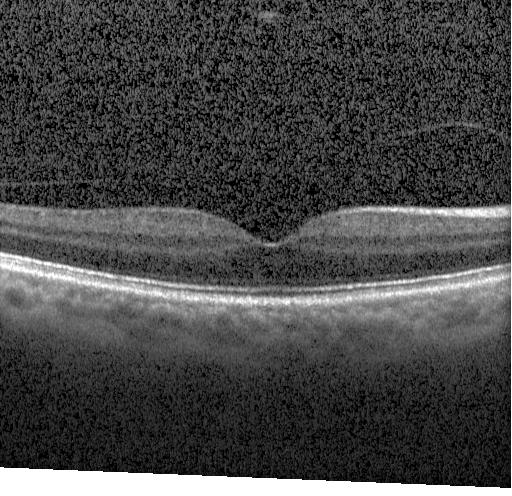

Finding: neither choroidal neovascularization, diabetic macular edema, nor drusen.